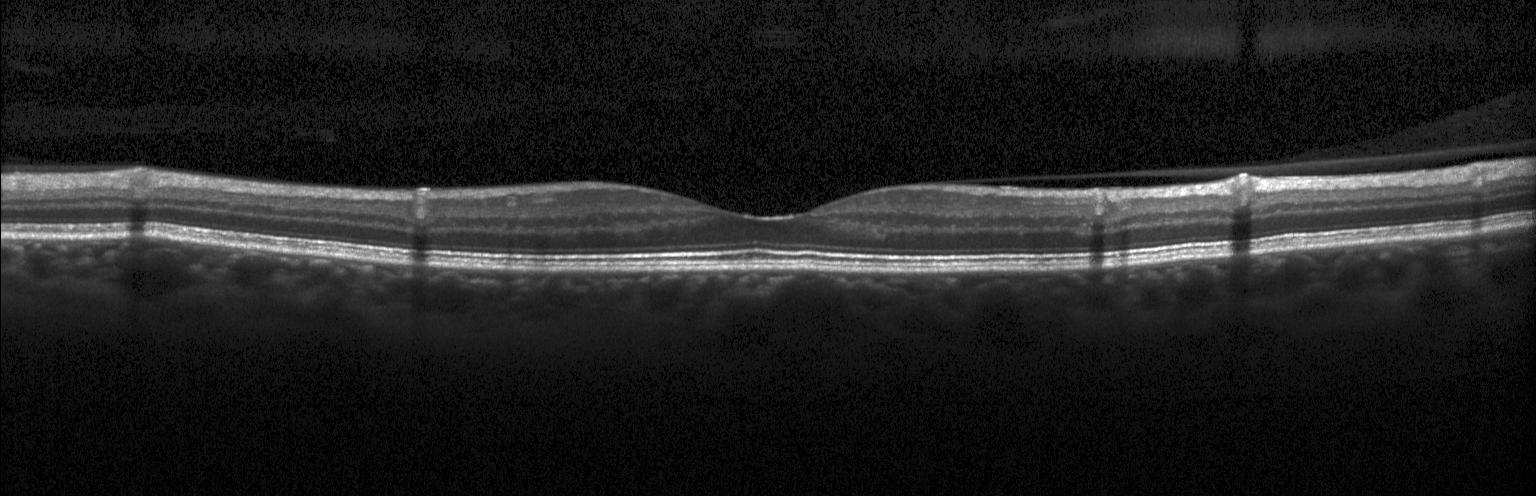

Macular OCT: no CNV, DME, or drusen.